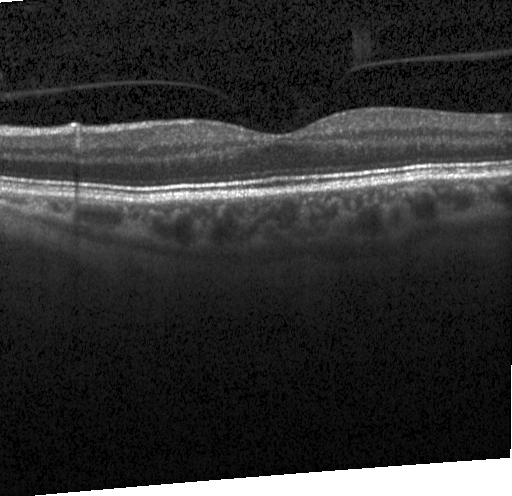
Assessment: no evidence of CNV, DME, or drusen.